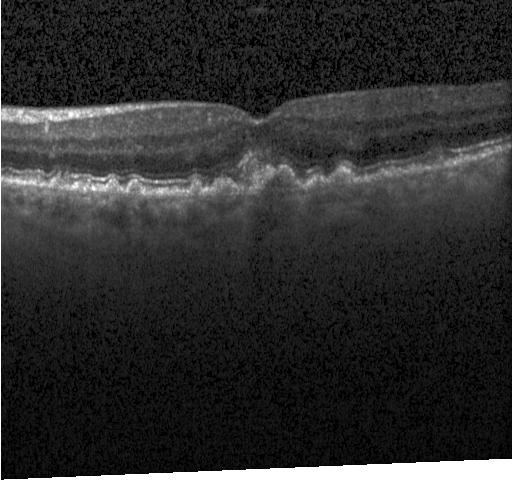 OCT line scan. Horizontal scan through the fovea. Spectral-domain OCT. Heidelberg Spectralis OCT system
Diagnosis: a choroidal neovascular membrane.